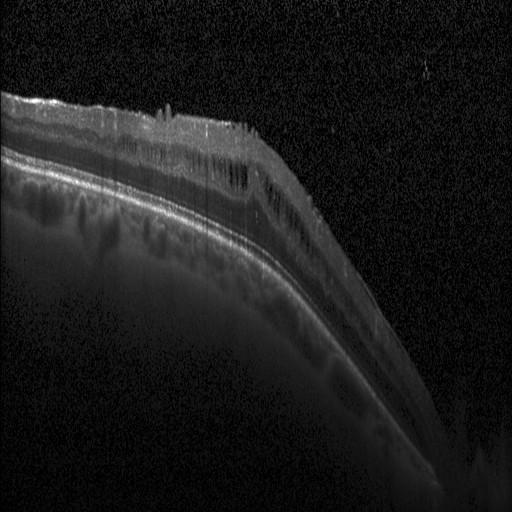 Retinal OCT B-scan; Heidelberg Spectralis OCT system; spectral-domain optical coherence tomography — Impression: DME.